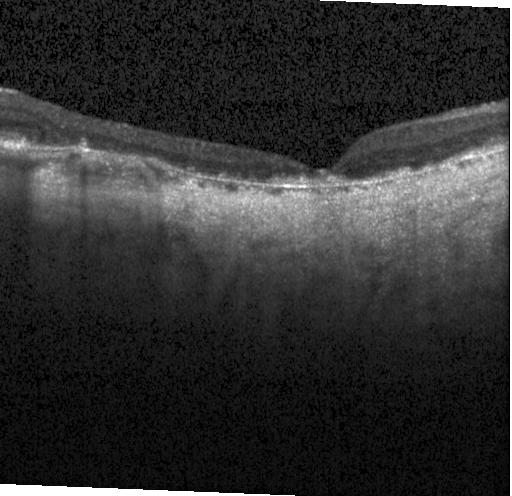 OCT B-scan — OCT finding: CNV.